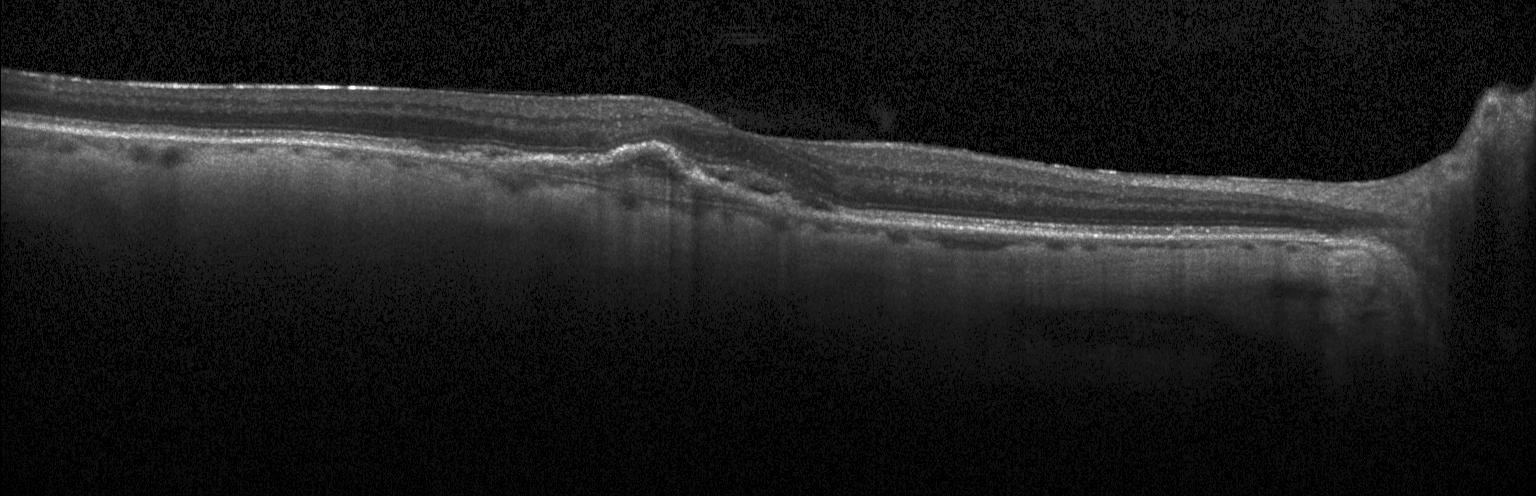

Impression: CNV.